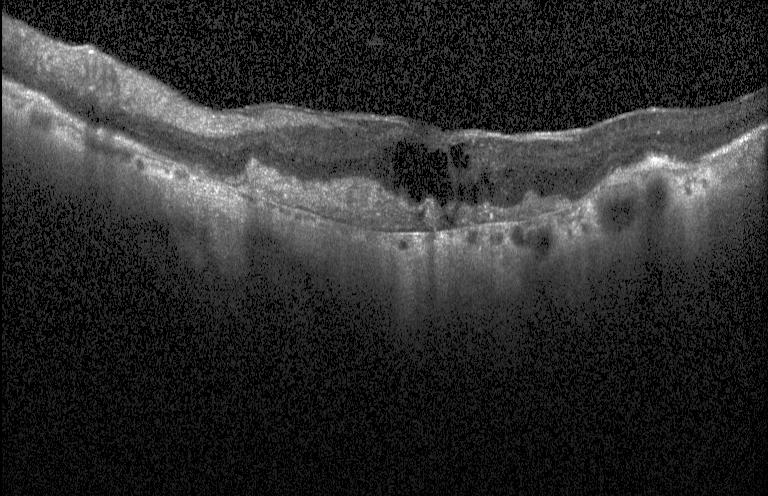 Macular OCT: a choroidal neovascular membrane.